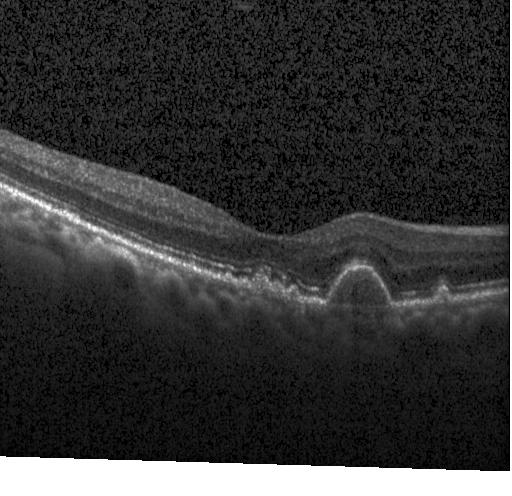

Optical coherence tomography scan · macular scan · SD-OCT · Heidelberg Spectralis — The scan shows sub-RPE drusenoid deposits.